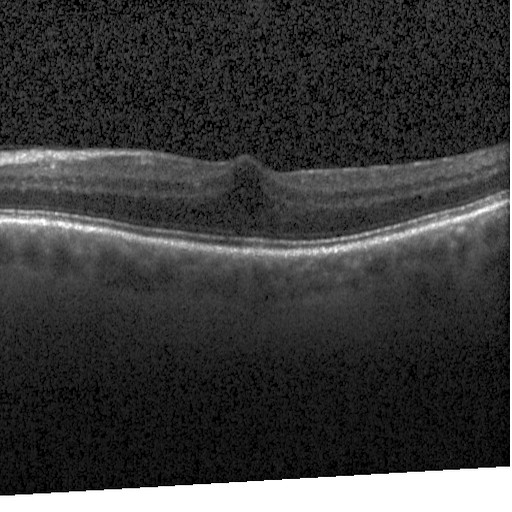

Heidelberg Spectralis OCT system; through the macula; retinal OCT B-scan; spectral-domain OCT.
Diagnosis: diabetic macular edema.